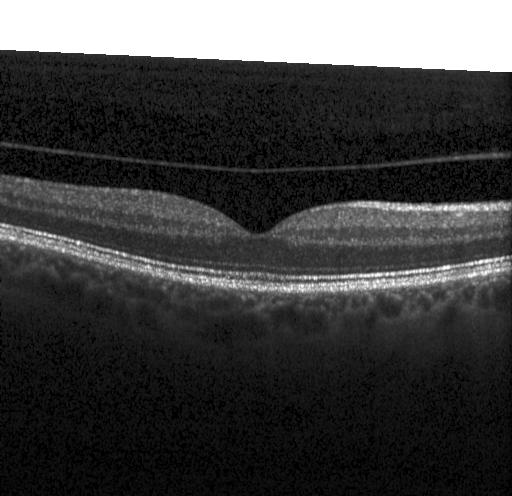 Horizontal scan through the fovea · optical coherence tomography B-scan · instrument: Heidelberg Spectralis · SD-OCT. No CNV, no DME, and no drusen.